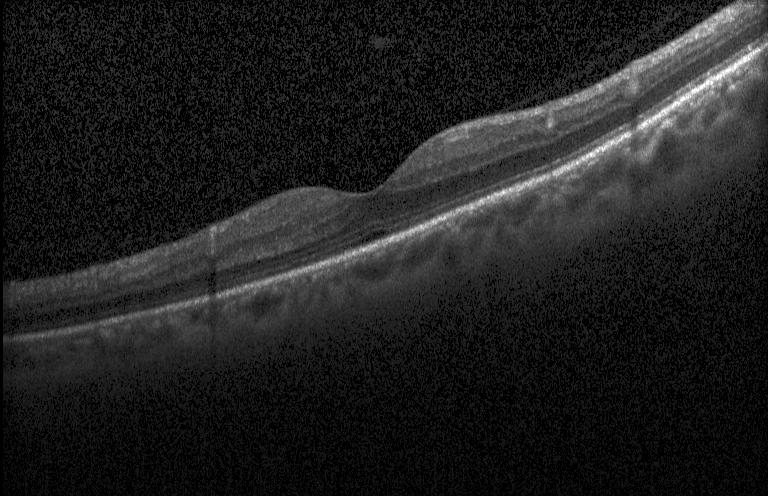
Optical coherence tomography scan · centered on the fovea · spectral-domain optical coherence tomography · Heidelberg Spectralis OCT system. This B-scan demonstrates no evidence of CNV, DME, or drusen.